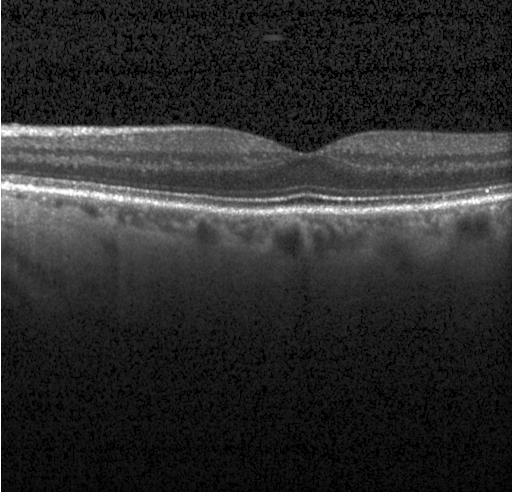

Optical coherence tomography scan · macular scan · spectral-domain OCT · instrument: Heidelberg Spectralis.
Diagnosis: neither choroidal neovascularization, diabetic macular edema, nor drusen.